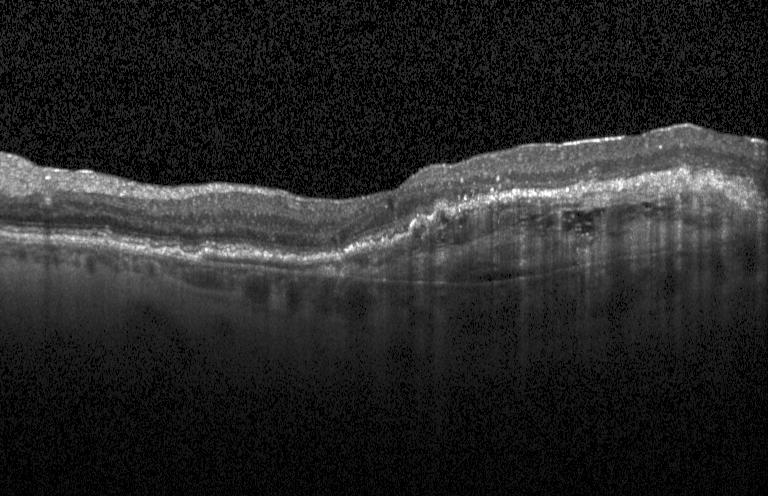

OCT B-scan. Instrument: Heidelberg Spectralis. Diagnosis: CNV.